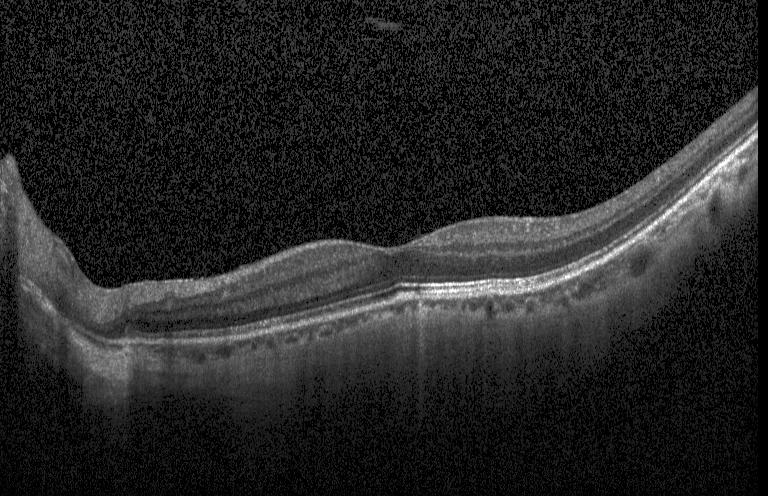
No evidence of choroidal neovascularization, diabetic macular edema, or drusen.